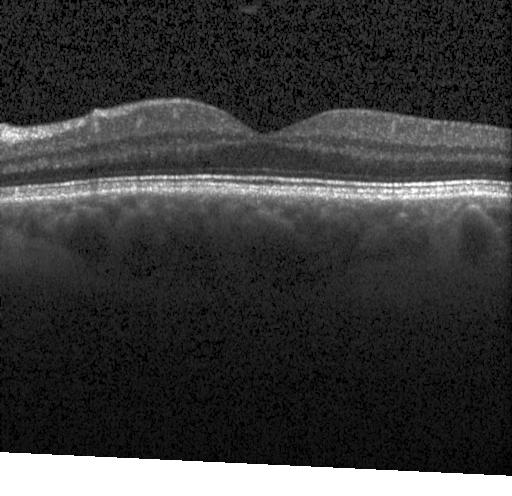

OCT B-scan.
The scan shows no choroidal neovascularization, no diabetic macular edema, and no drusen.